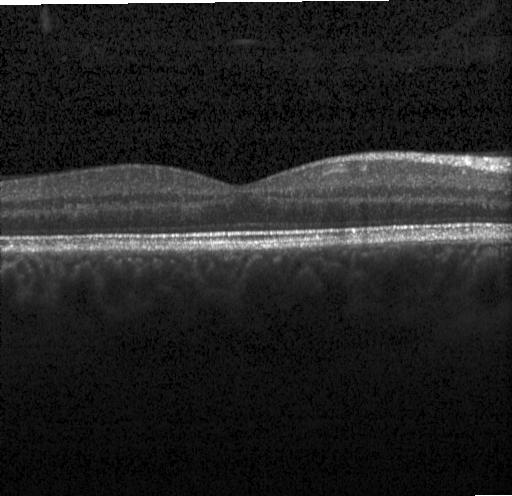
Finding: no evidence of CNV, DME, or drusen.